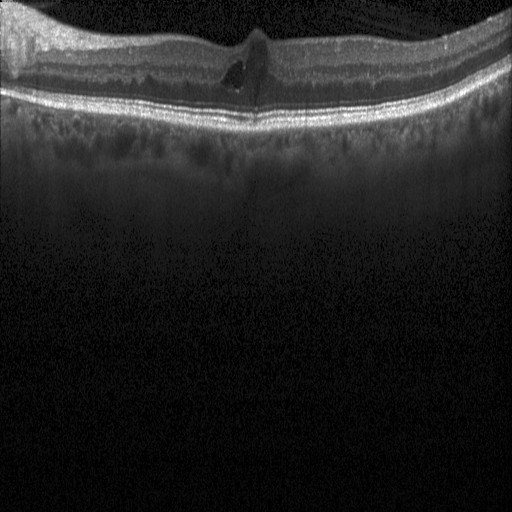 Finding: DME.